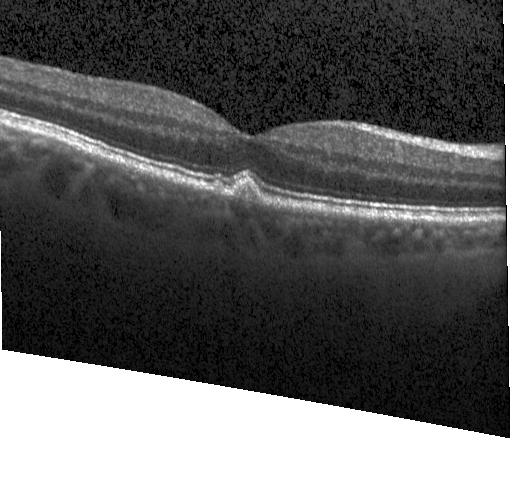 OCT B-scan.
Multiple drusen.